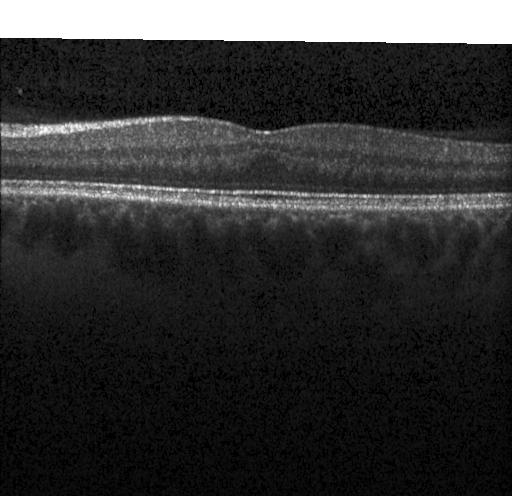
Diagnosis: no evidence of choroidal neovascularization, diabetic macular edema, or drusen.